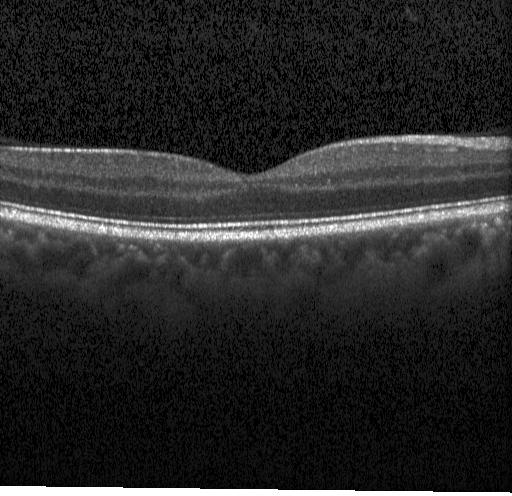
Diagnosis: neither CNV, DME, nor drusen.